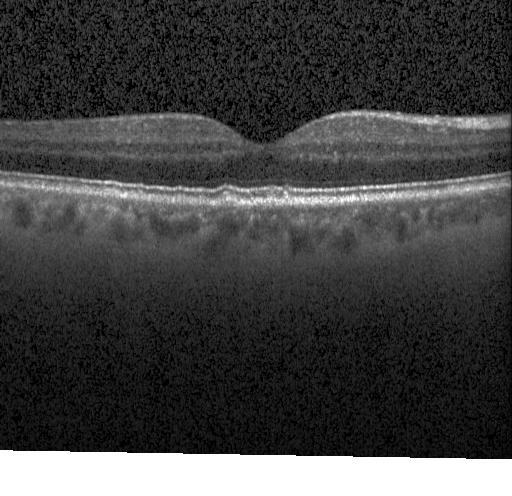 OCT B-scan.
Finding: drusen.